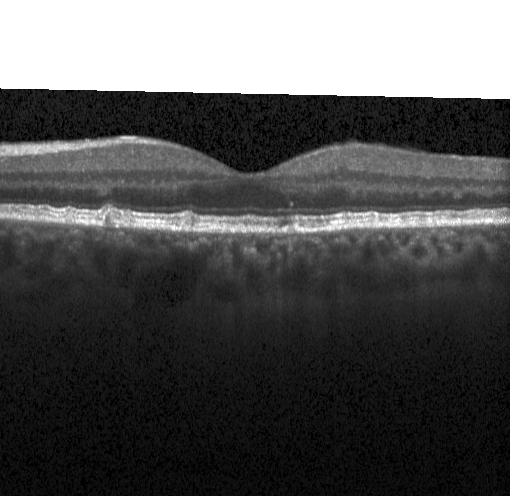
Optical coherence tomography B-scan. Horizontal scan through the fovea.
Finding: drusen.